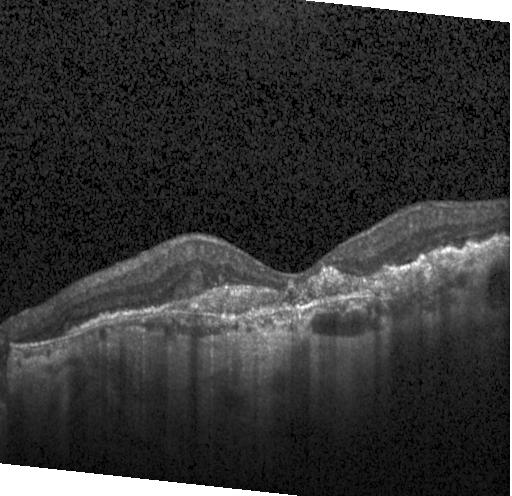

Retinal OCT cross-section. This B-scan demonstrates CNV.